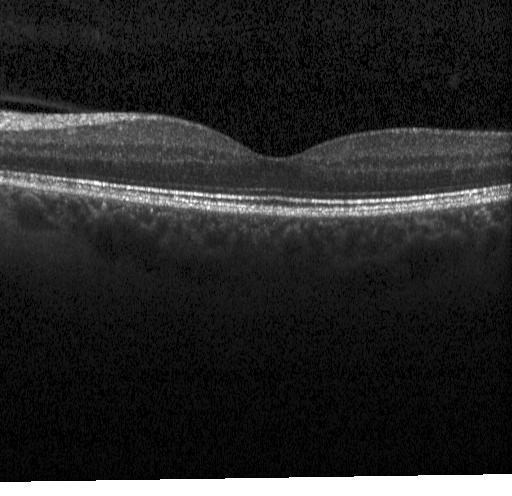 Retinal OCT cross-section.
Diagnosis: no evidence of choroidal neovascularization, diabetic macular edema, or drusen.